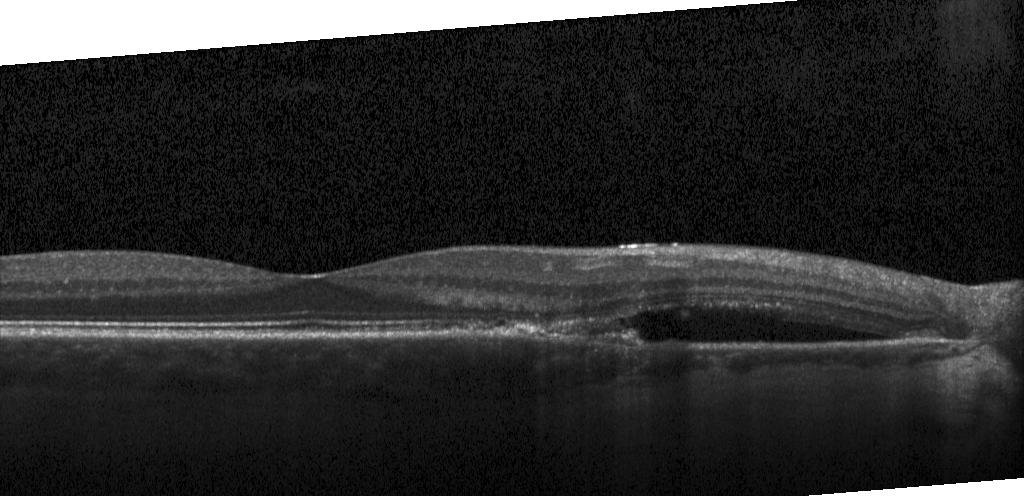
Choroidal neovascularization.